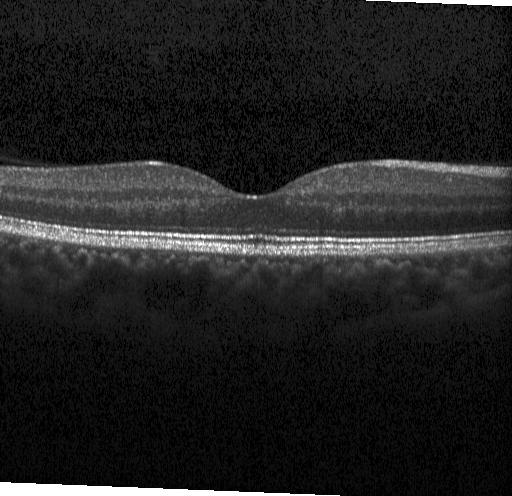 Acquired on a Heidelberg Spectralis, retinal OCT cross-section, horizontal scan through the fovea
OCT finding: no choroidal neovascularization, diabetic macular edema, or drusen.